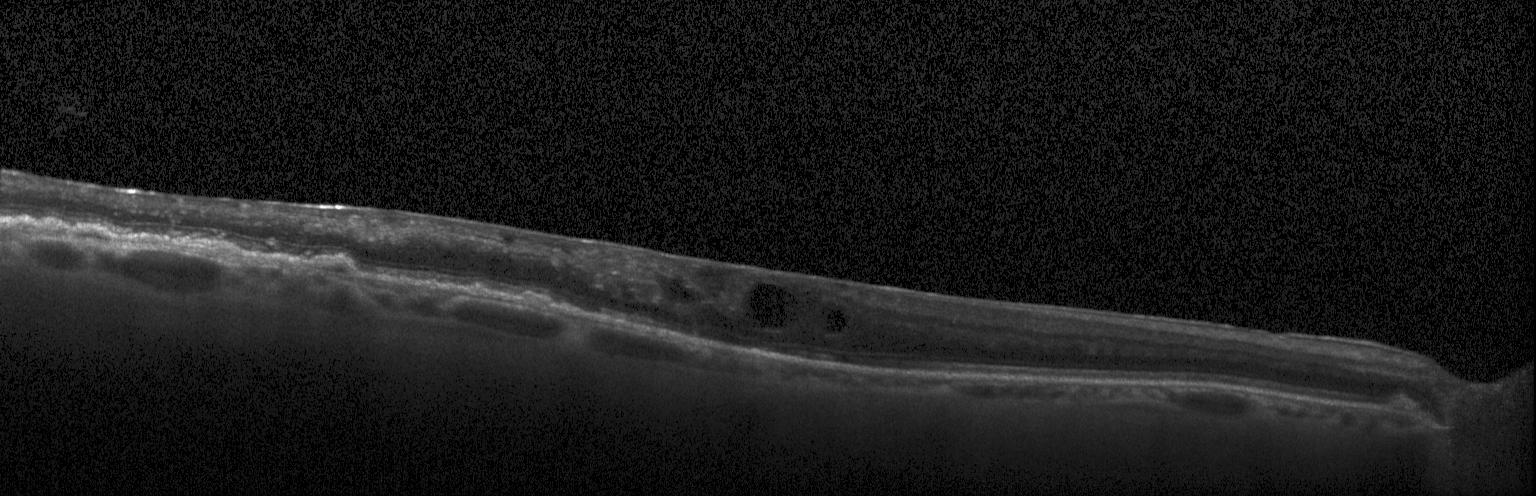

Optical coherence tomography scan
Impression: choroidal neovascularization (CNV).